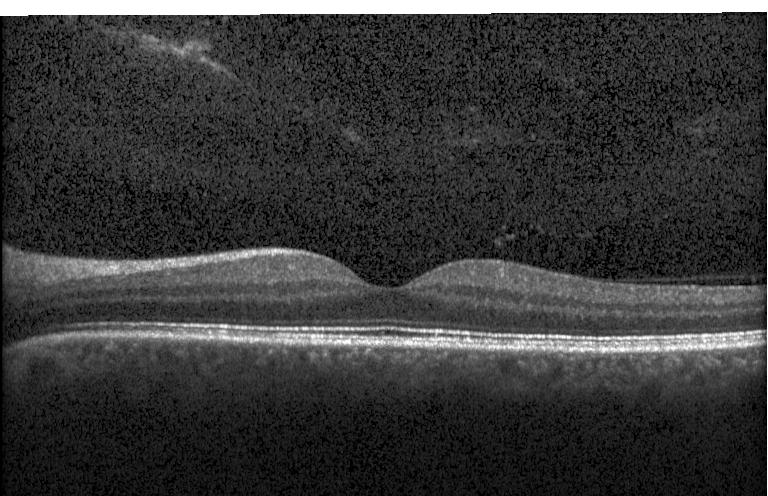 Optical coherence tomography scan. The scan shows no CNV, DME, or drusen.